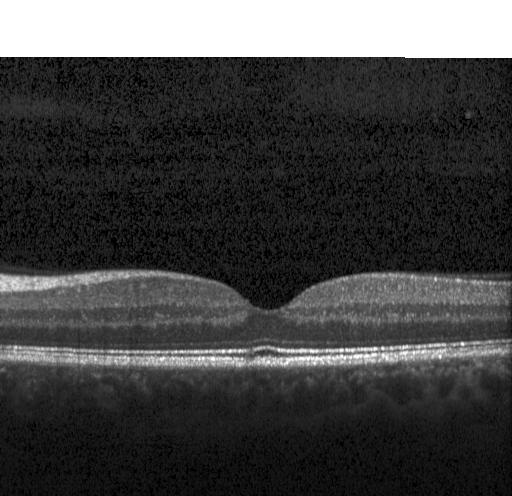 Impression: neither CNV, DME, nor drusen.